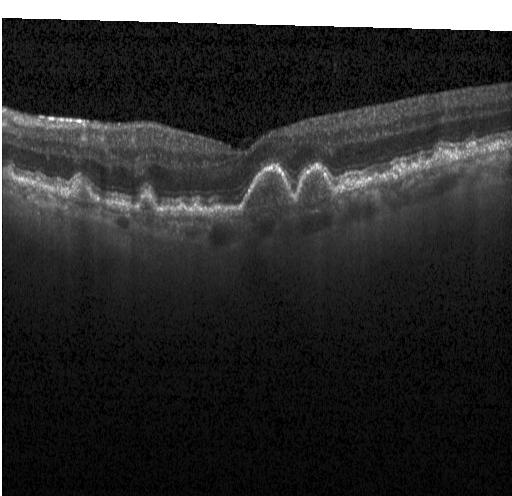

The scan shows sub-RPE drusenoid deposits.